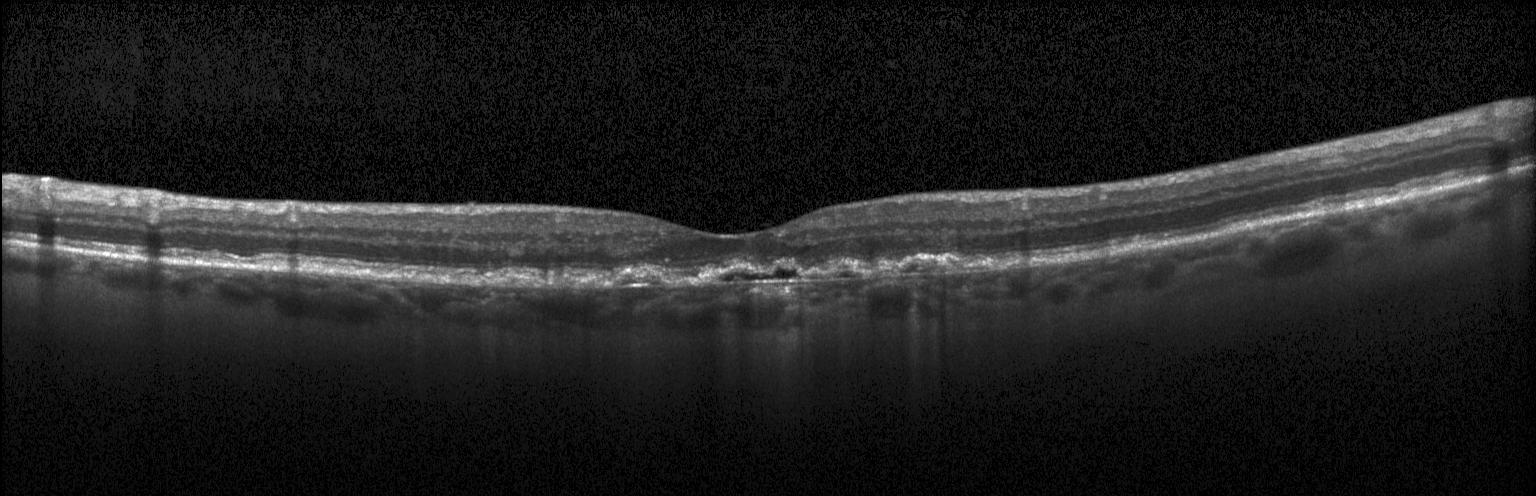 A choroidal neovascular membrane.